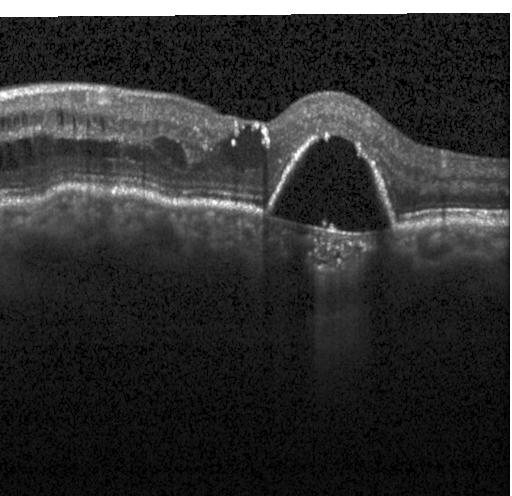

Retinal OCT cross-section showing a choroidal neovascular membrane.